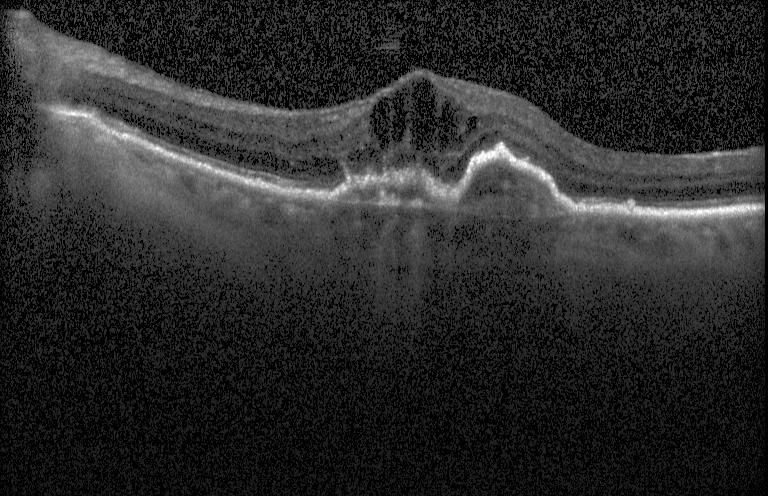

Finding: choroidal neovascularization (CNV).